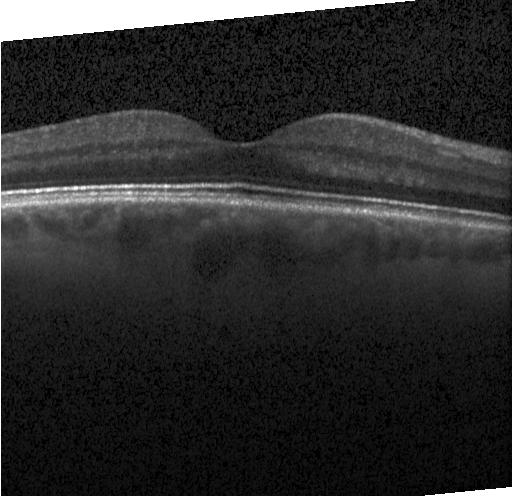
SD-OCT; OCT line scan. Macular OCT: no evidence of CNV, DME, or drusen.